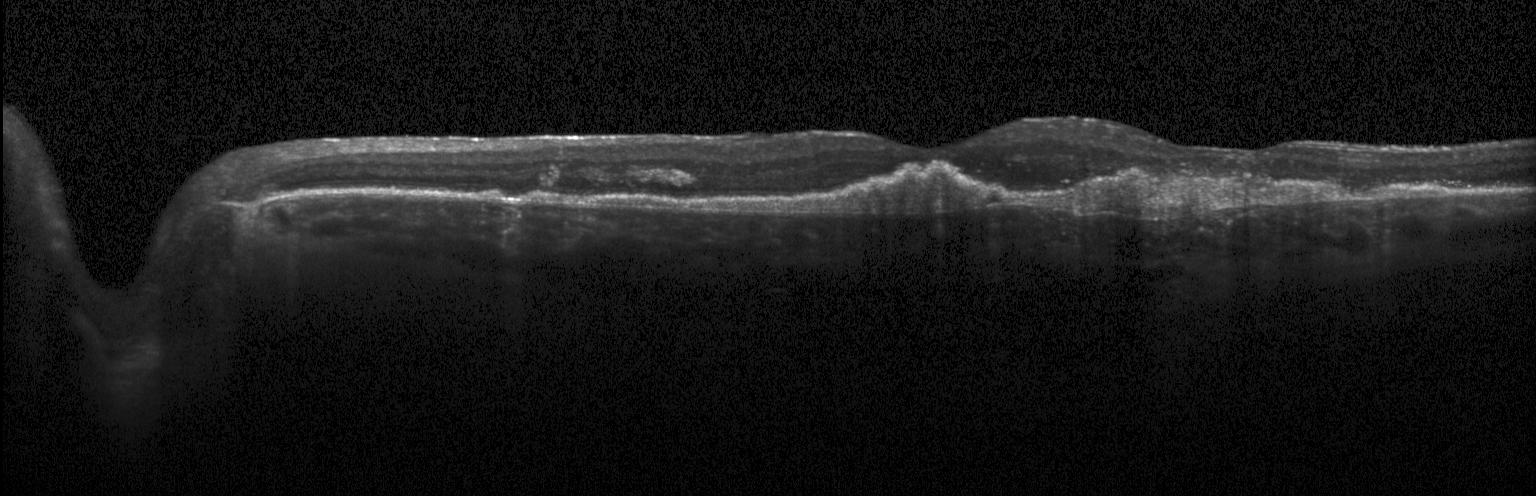

Spectral-domain OCT B-scan: CNV.